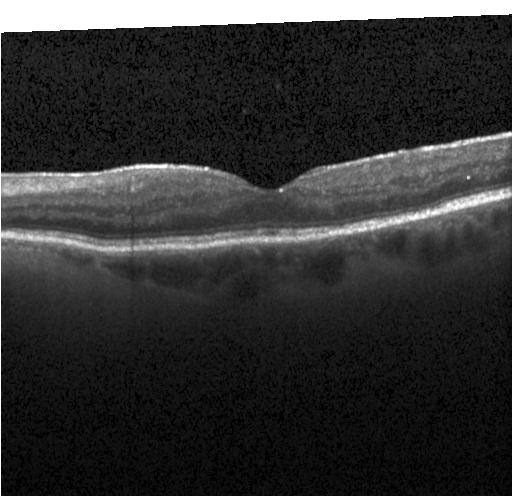
Optical coherence tomography B-scan. Finding: no choroidal neovascularization, no diabetic macular edema, and no drusen.